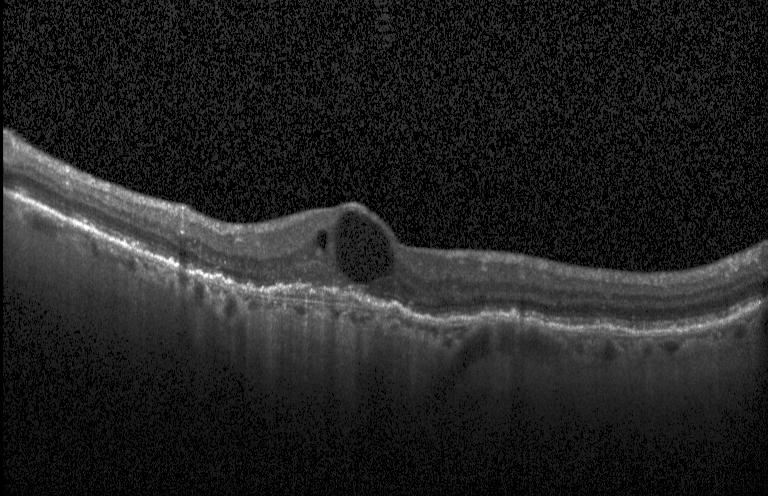 Optical coherence tomography B-scan.
Assessment: a choroidal neovascular membrane.